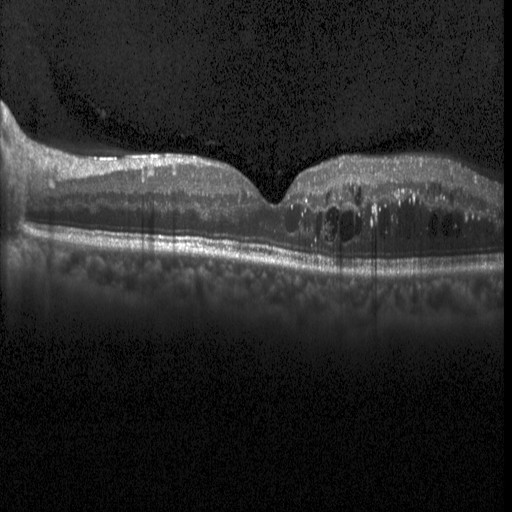
Macular OCT demonstrating diabetic macular edema.